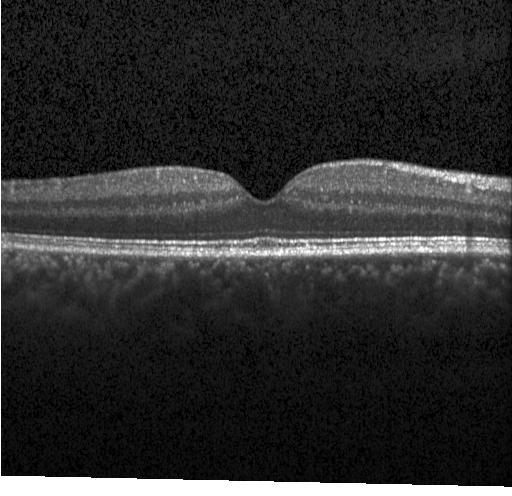
OCT line scan. Diagnosis: no CNV, no DME, and no drusen.